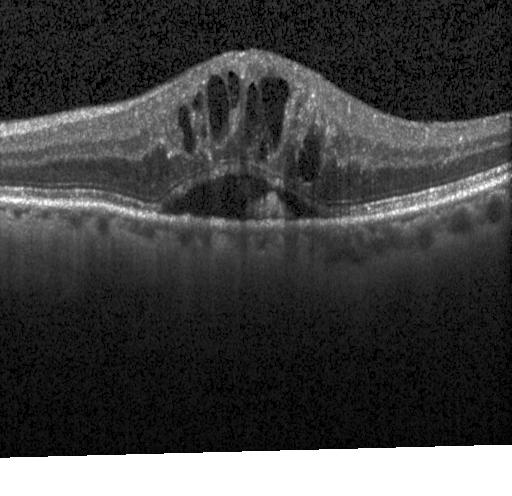

SD-OCT · Heidelberg Spectralis OCT system · retinal OCT cross-section
Assessment: diabetic macular edema (DME).